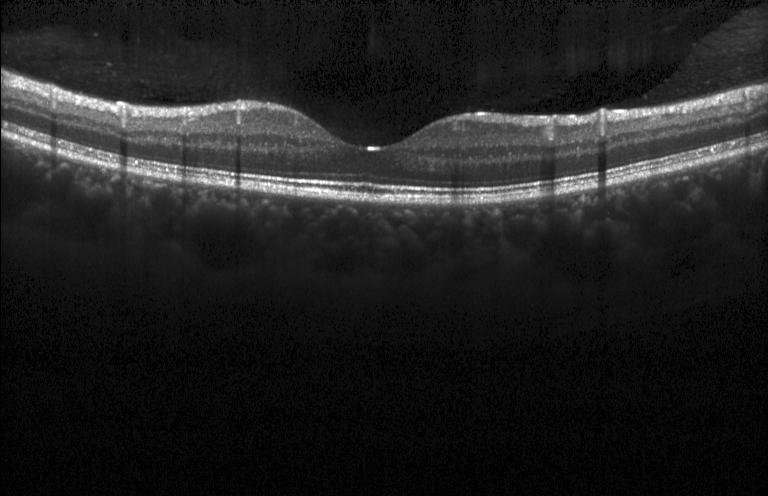

Through the macula. OCT B-scan. Spectral-domain optical coherence tomography — OCT finding: no evidence of CNV, DME, or drusen.